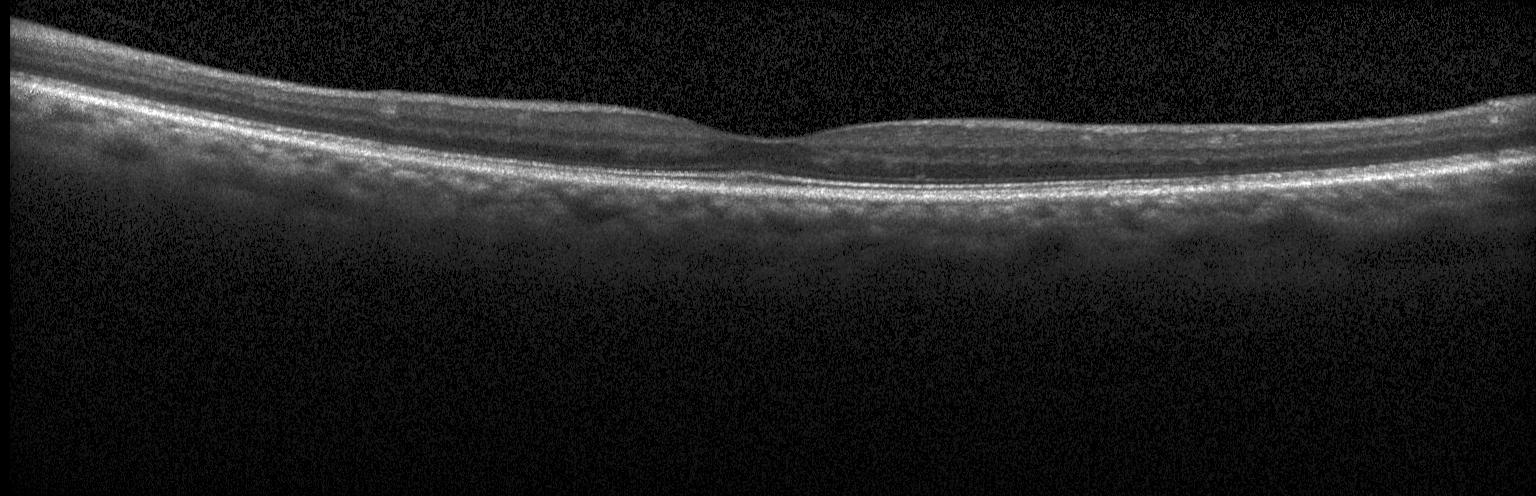
Retinal OCT cross-section — OCT finding: no evidence of CNV, DME, or drusen.